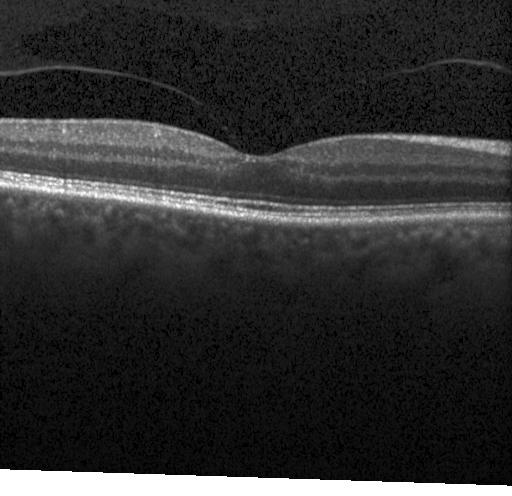

OCT finding: no choroidal neovascularization, diabetic macular edema, or drusen.